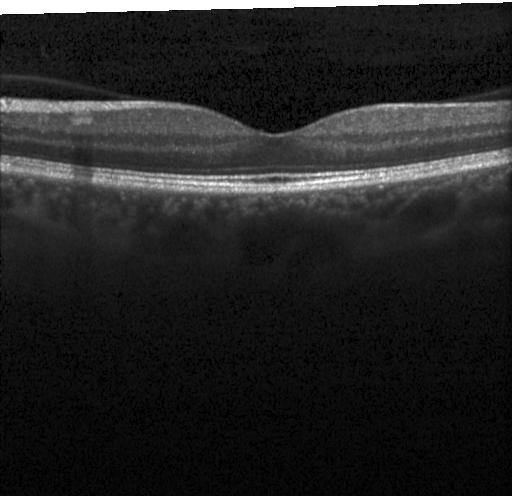

Finding: neither choroidal neovascularization, diabetic macular edema, nor drusen.